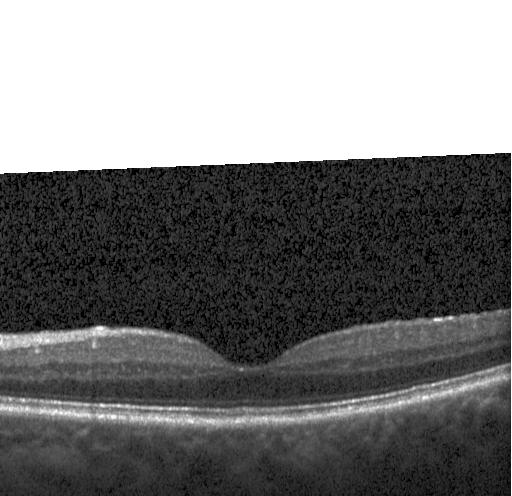

Retinal OCT cross-section. Acquired on a Heidelberg Spectralis. Fovea-centered — The scan shows no CNV, no DME, and no drusen.